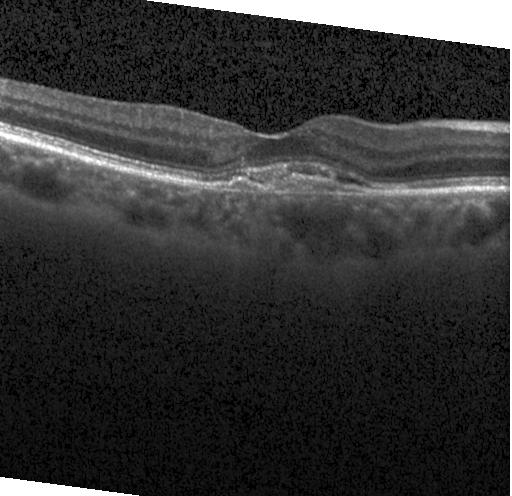

Dx: choroidal neovascularization.